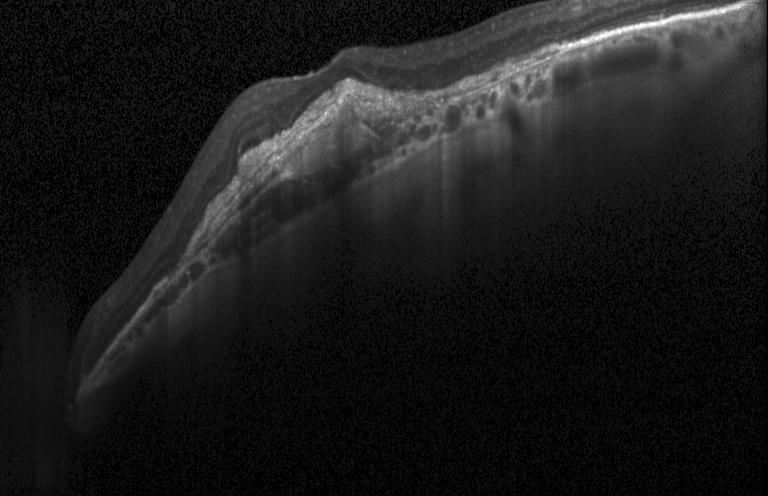

Optical coherence tomography scan
Diagnosis: CNV.